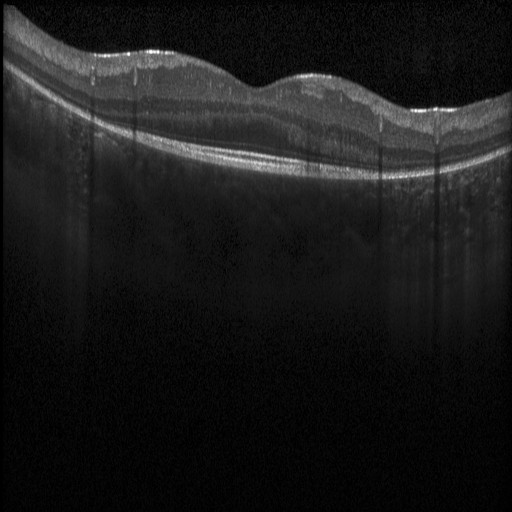
Instrument: Heidelberg Spectralis. Optical coherence tomography B-scan. Centered on the fovea. Spectral-domain OCT
The scan shows diabetic macular edema (DME).